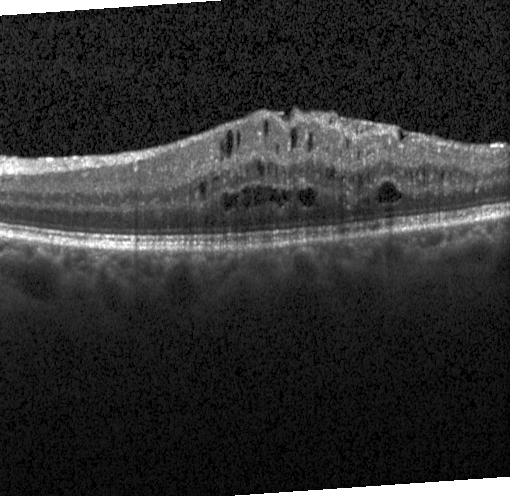
Finding: DME.